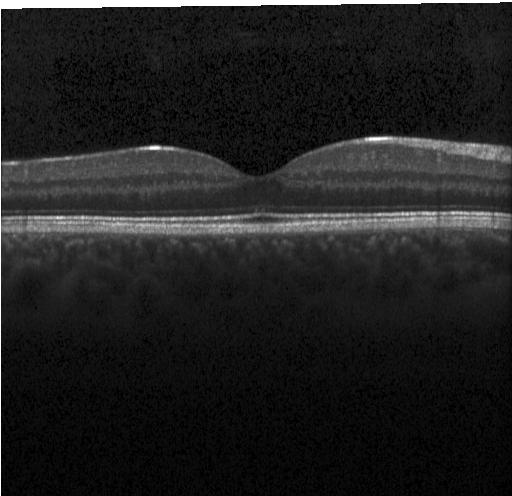
The scan shows neither choroidal neovascularization, diabetic macular edema, nor drusen.